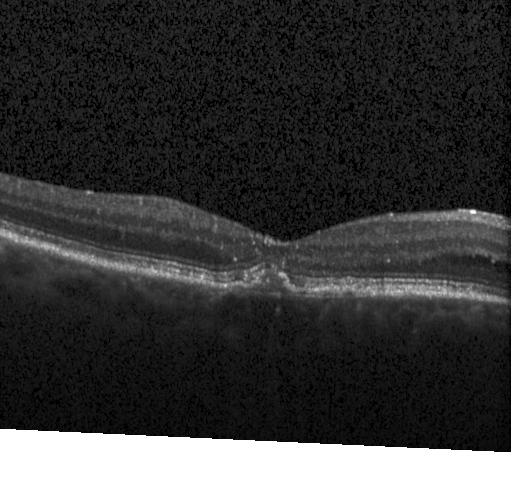 Retinal OCT B-scan.
Diagnosis: CNV.